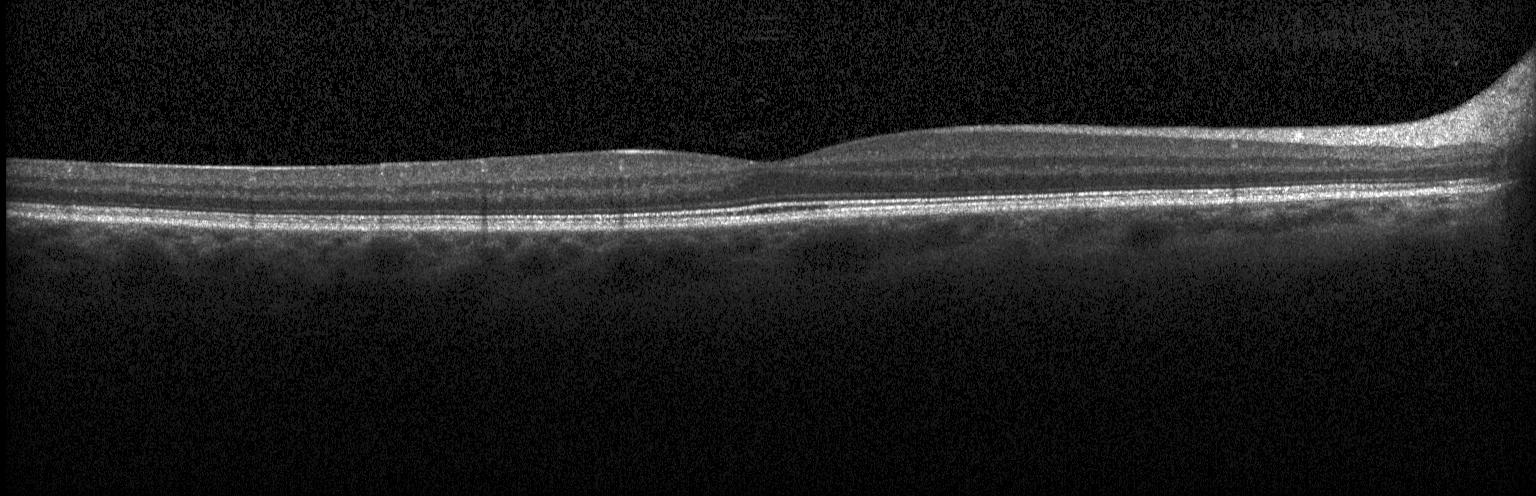
OCT line scan.
Diagnosis: no choroidal neovascularization, no diabetic macular edema, and no drusen.